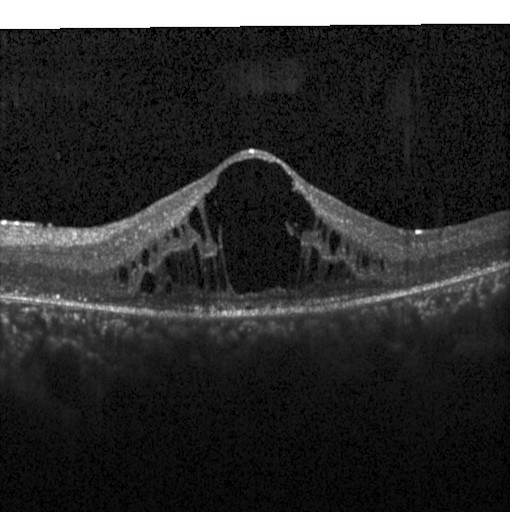

Spectral-domain OCT; retinal OCT cross-section — Assessment: diabetic macular edema (DME).